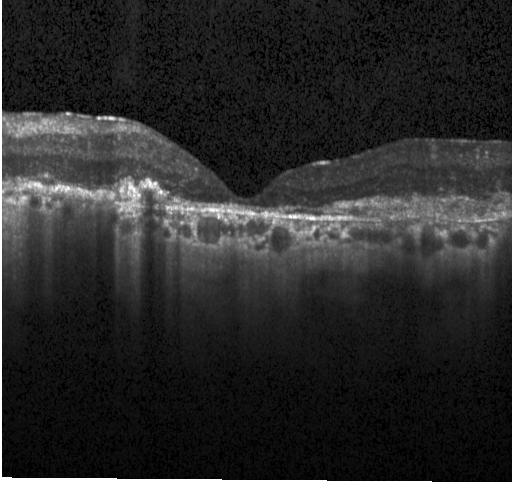

Retinal OCT B-scan — Assessment: CNV.